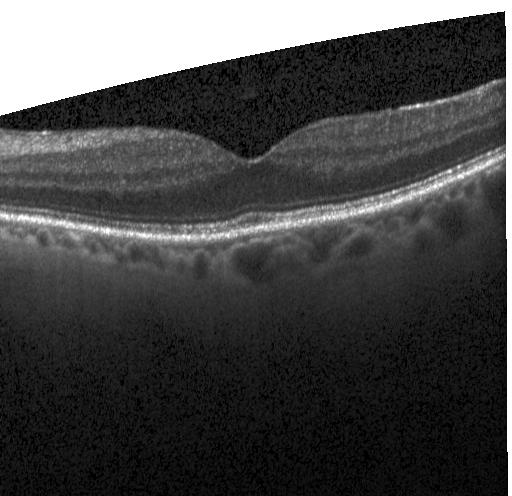

Finding: neither CNV, DME, nor drusen.